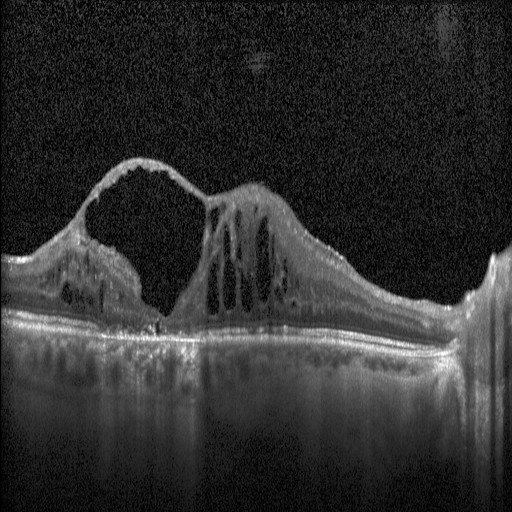 Macular scan. Optical coherence tomography B-scan — Finding: diabetic macular edema (DME).